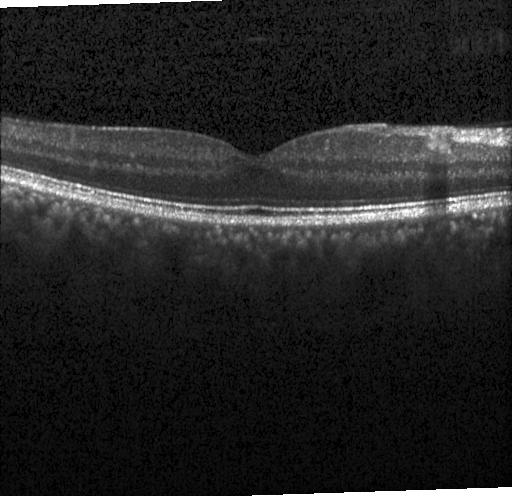

OCT B-scan, horizontal scan through the fovea, SD-OCT, acquired on a Heidelberg Spectralis. Neither choroidal neovascularization, diabetic macular edema, nor drusen.